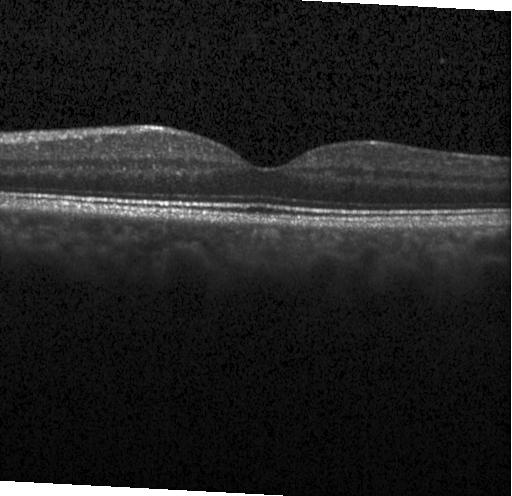
Retinal OCT cross-section — Impression: no CNV, DME, or drusen.